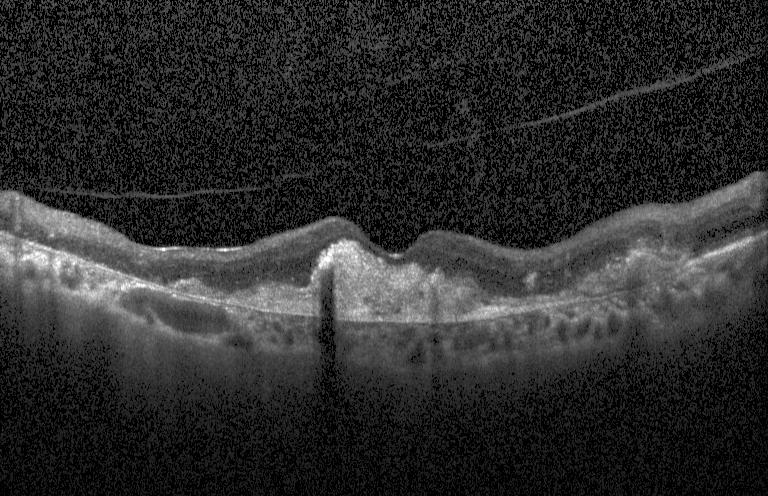
Impression: choroidal neovascularization.